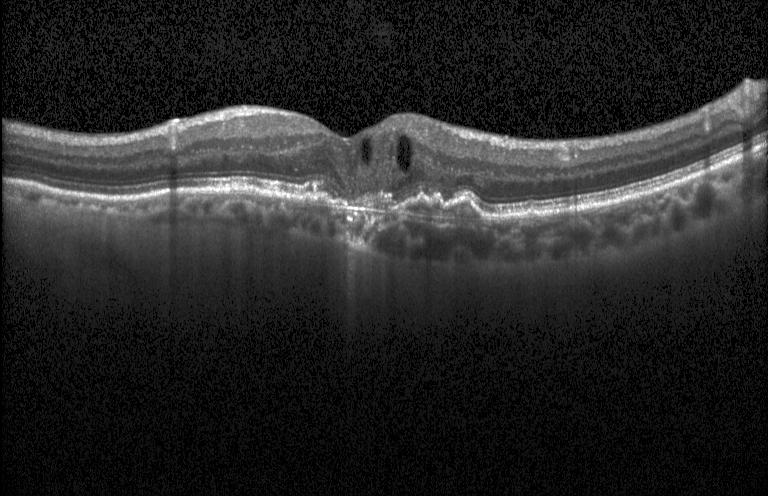

Spectral-domain OCT · retinal OCT cross-section · acquired on a Heidelberg Spectralis · fovea-centered.
Dx: choroidal neovascularization.